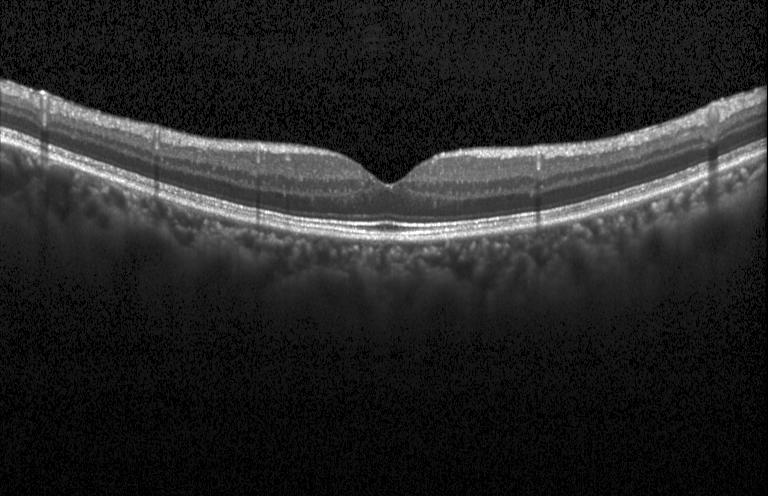

Macular OCT: no choroidal neovascularization, no diabetic macular edema, and no drusen.